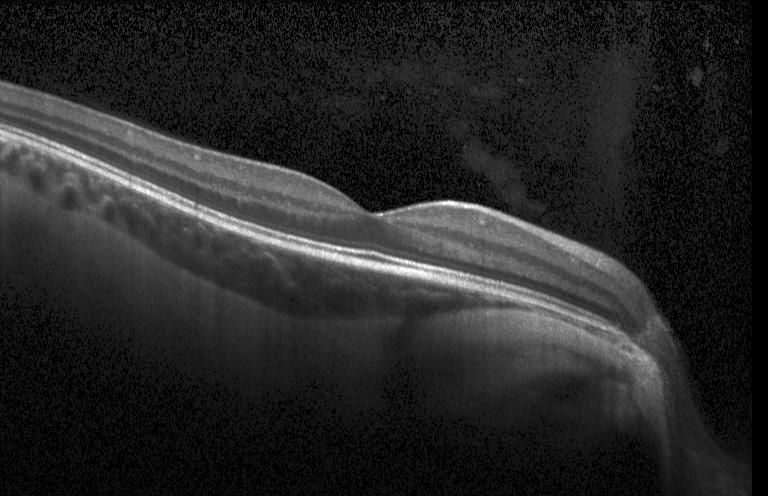

Macular scan. OCT line scan. SD-OCT. Heidelberg Spectralis OCT system
Impression: no choroidal neovascularization, diabetic macular edema, or drusen.